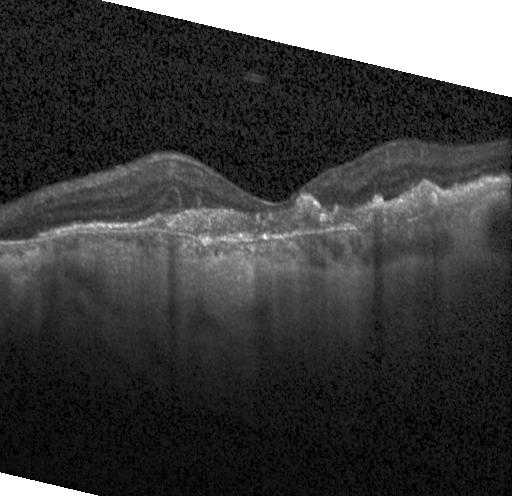
OCT scan showing a choroidal neovascular membrane.